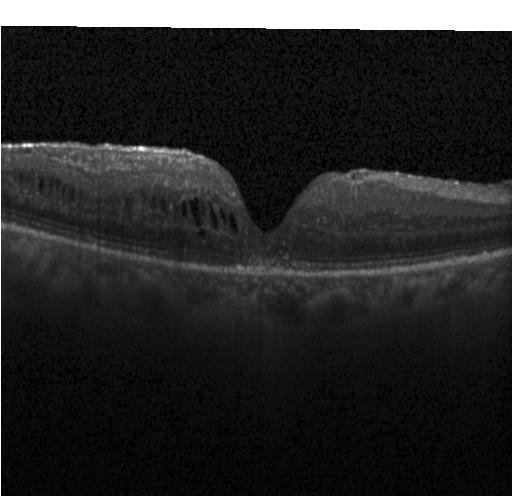 Retinal OCT cross-section · spectral-domain optical coherence tomography.
Diagnosis: diabetic macular edema.